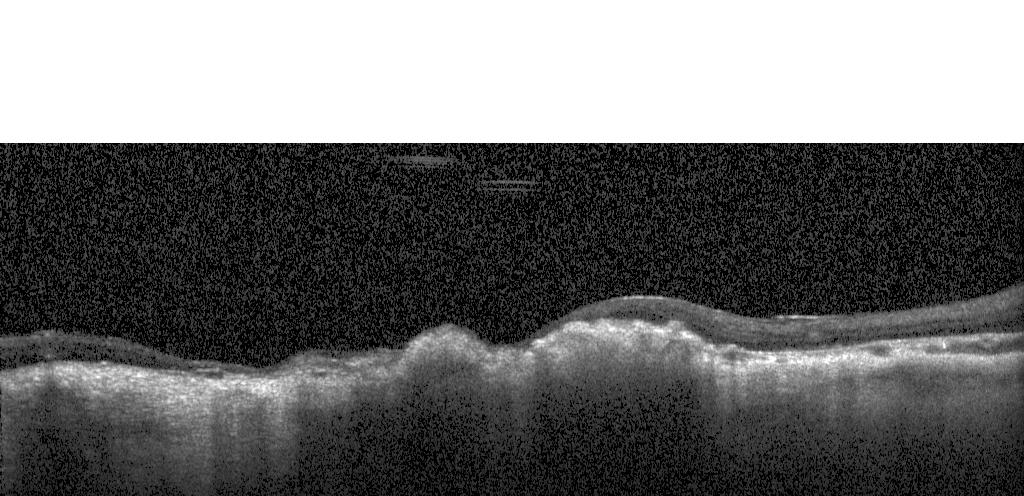
Macular OCT: CNV.